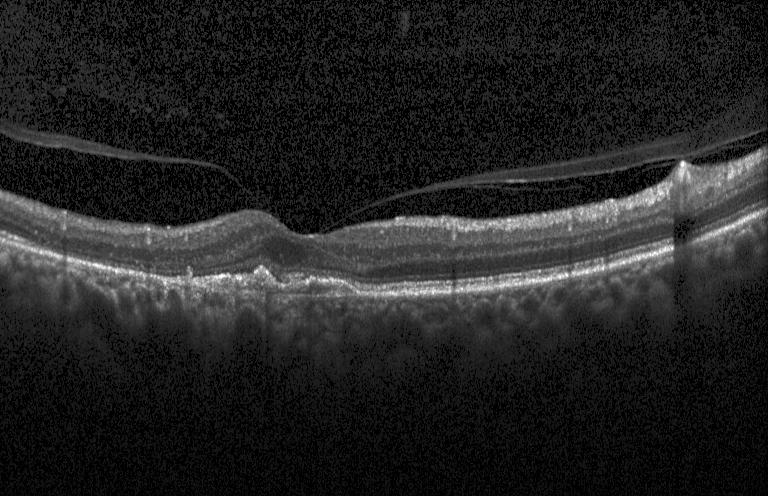
Optical coherence tomography scan · spectral-domain OCT · horizontal scan through the fovea · acquired on a Heidelberg Spectralis. This B-scan demonstrates choroidal neovascularization (CNV).